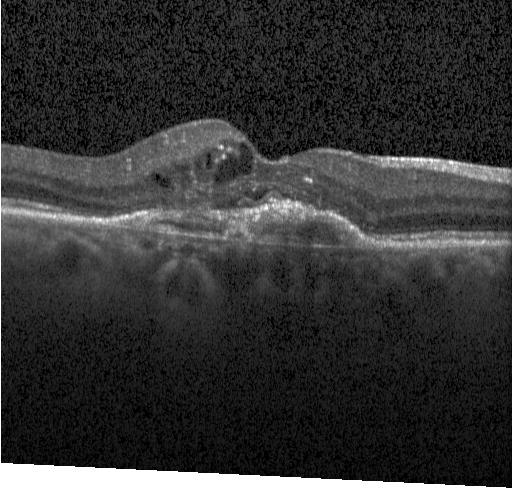

Diagnosis: CNV.